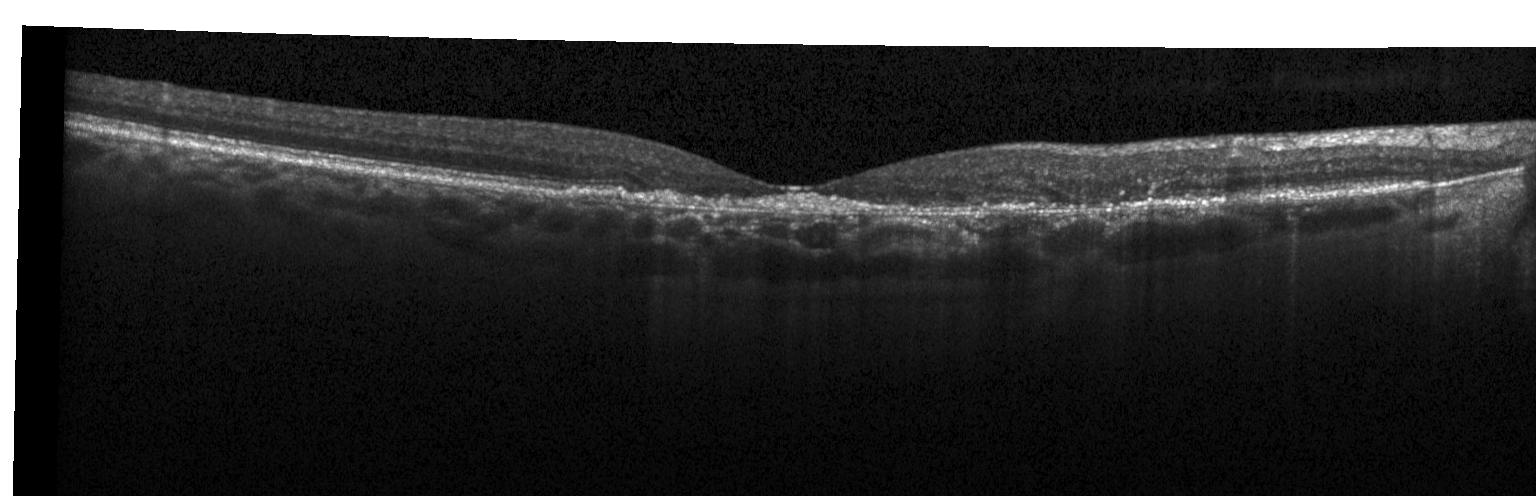 Retinal OCT cross-section · macular scan. Dx: choroidal neovascularization.